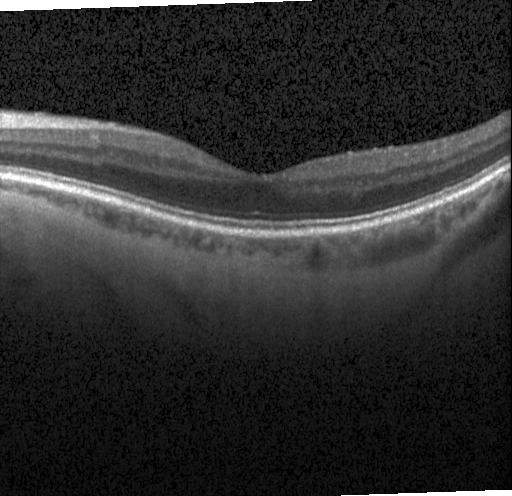
Optical coherence tomography scan; SD-OCT; instrument: Heidelberg Spectralis — Diagnosis: no evidence of CNV, DME, or drusen.